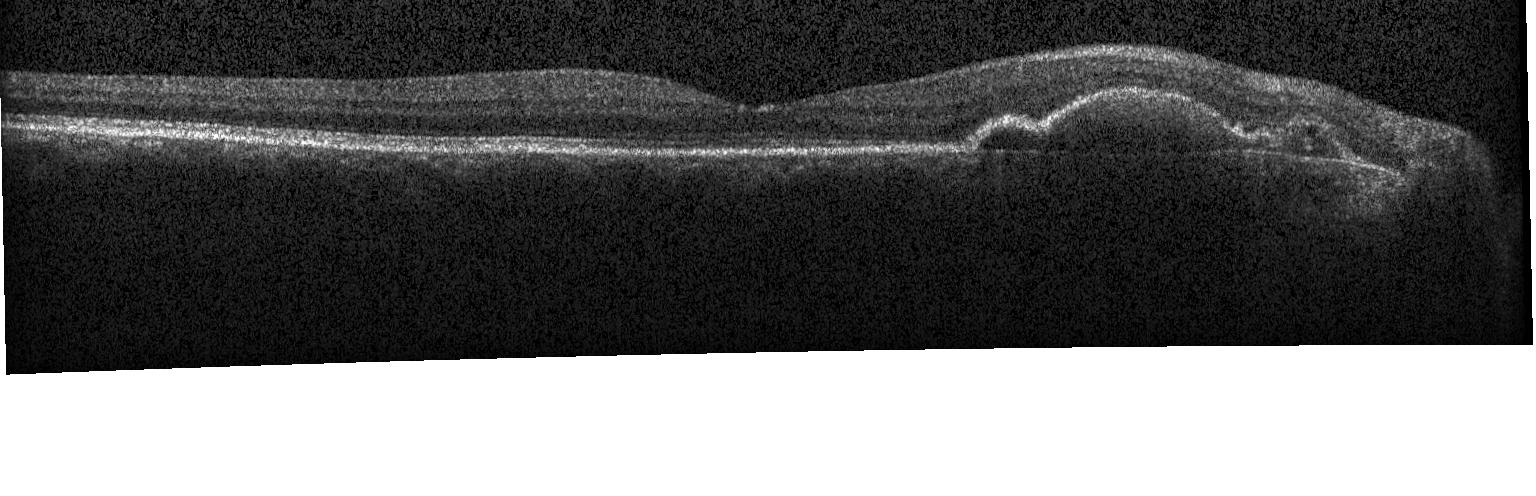

Macular OCT demonstrating choroidal neovascularization.